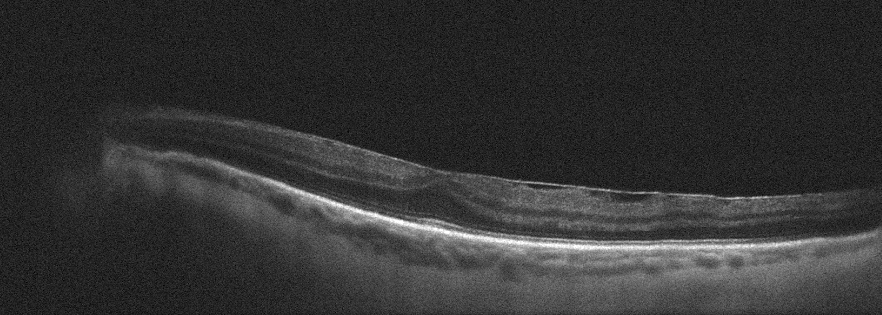 Instrument: Optovue Avanti RTVue XR; macular scan; retinal OCT B-scan
Assessment: epiretinal membrane.